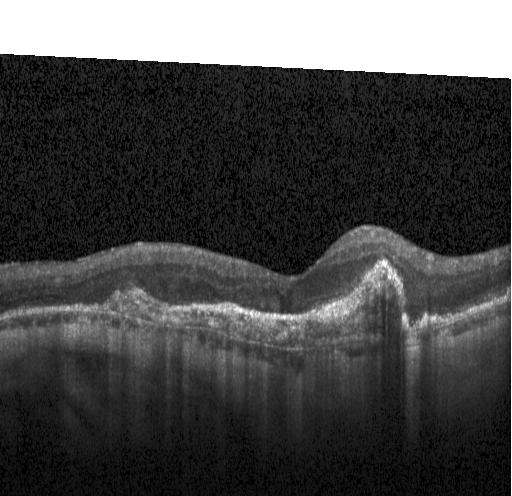 Spectral-domain OCT B-scan: choroidal neovascularization.